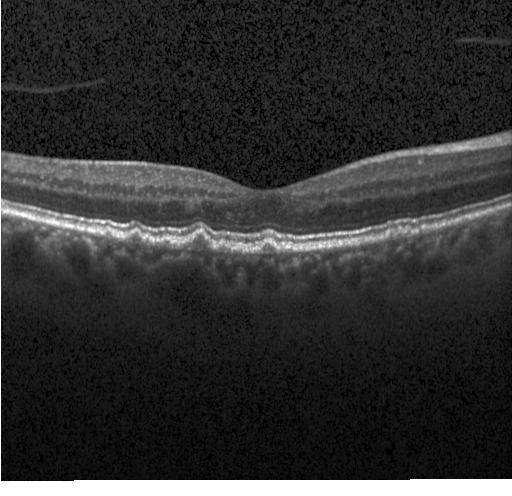 OCT B-scan showing multiple drusen.